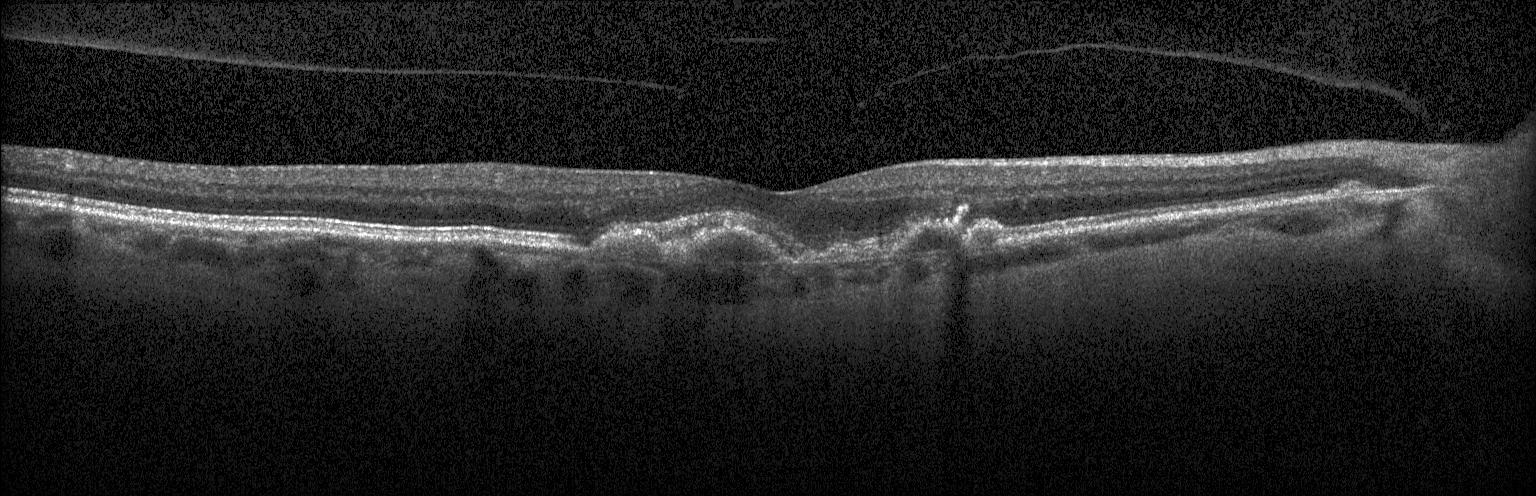

Diagnosis: a choroidal neovascular membrane.